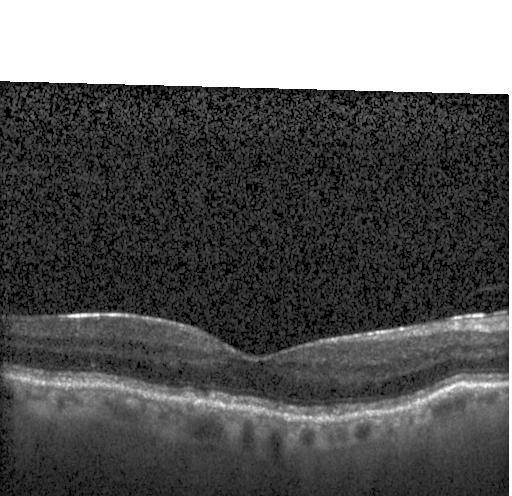 Spectral-domain OCT; retinal OCT B-scan; macular scan.
Finding: no choroidal neovascularization, diabetic macular edema, or drusen.